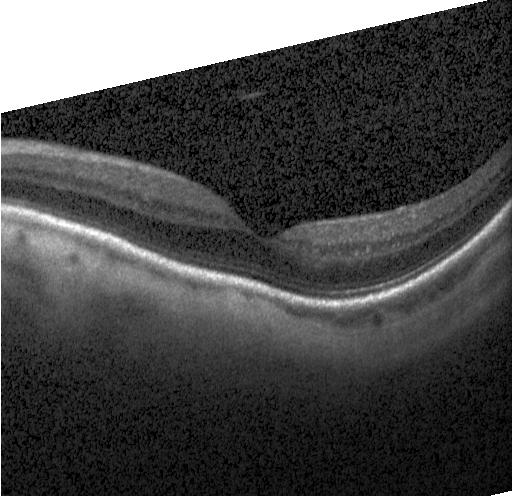
Optical coherence tomography scan; spectral-domain OCT. Impression: neither CNV, DME, nor drusen.